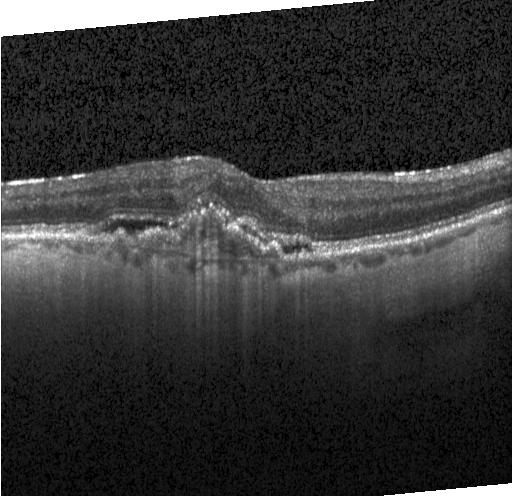 Retinal OCT cross-section, spectral-domain optical coherence tomography, Heidelberg Spectralis — Dx: a choroidal neovascular membrane.